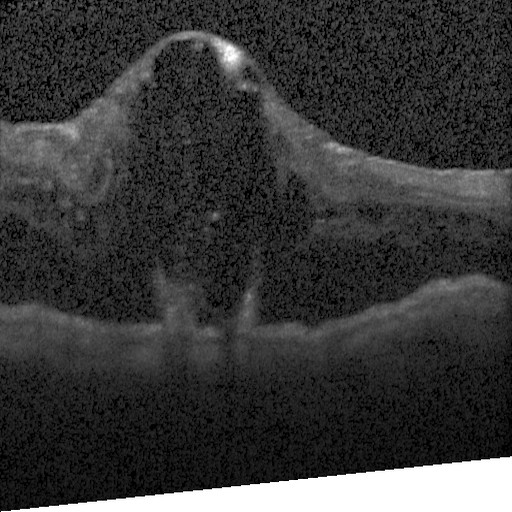

Retinal OCT cross-section showing DME.